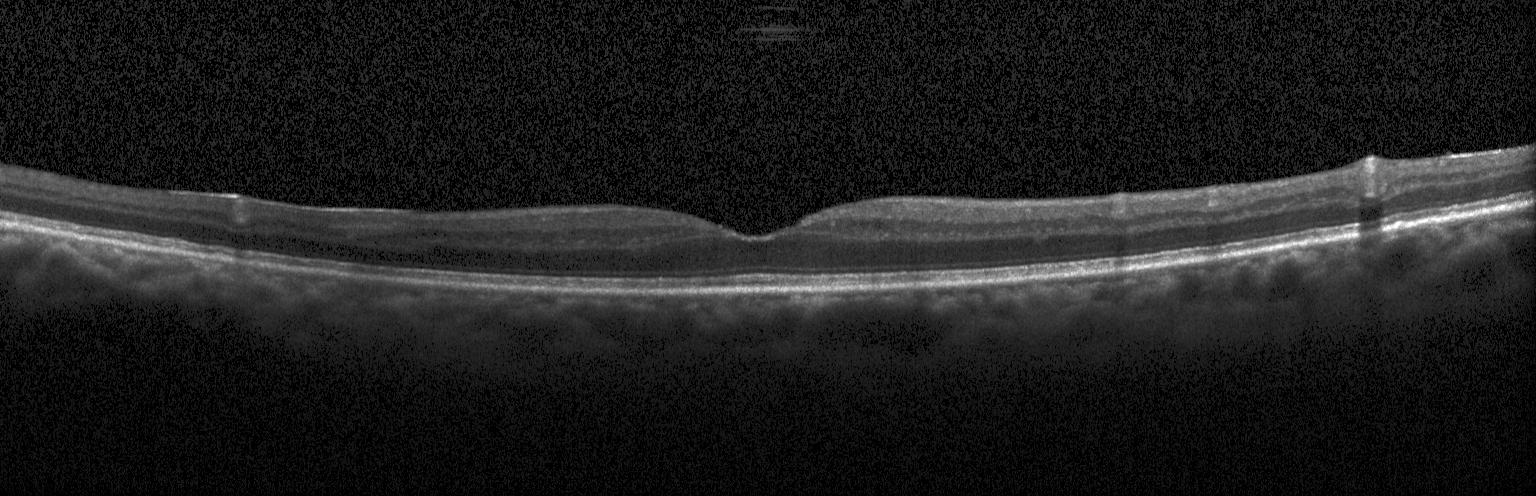
OCT B-scan. Diagnosis: no CNV, no DME, and no drusen.